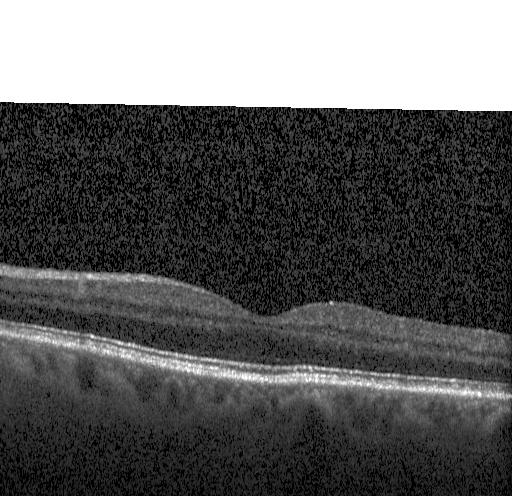
Spectral-domain optical coherence tomography. Instrument: Heidelberg Spectralis. Optical coherence tomography B-scan
OCT finding: no CNV, no DME, and no drusen.